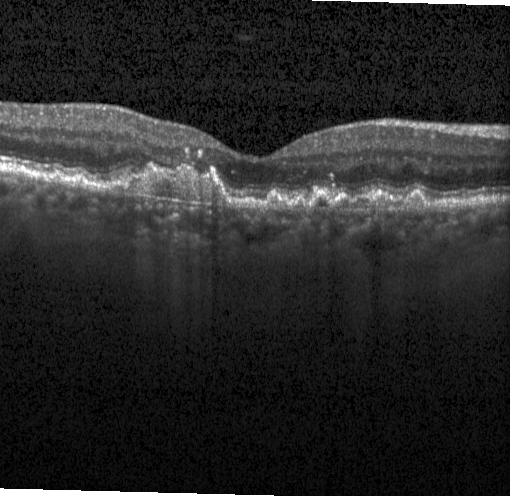

SD-OCT, optical coherence tomography B-scan.
Macular OCT: a choroidal neovascular membrane.